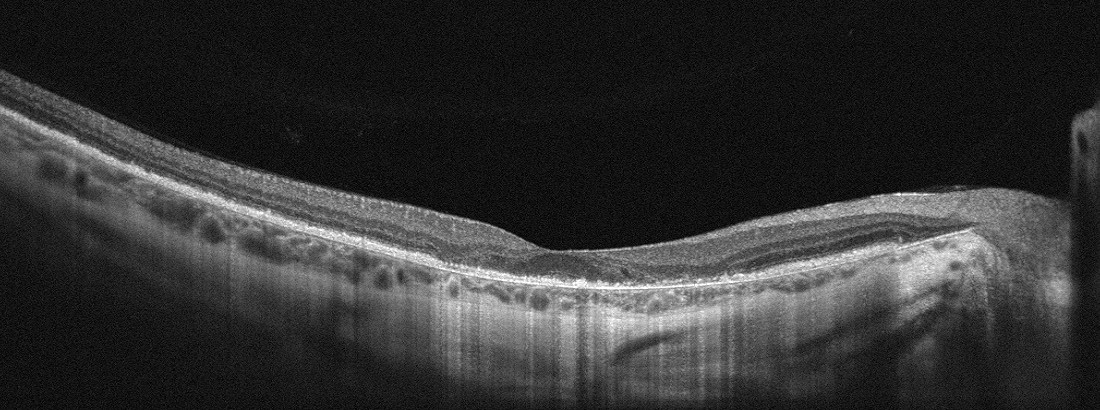
Retinal OCT B-scan.
Diagnosis: AMD.